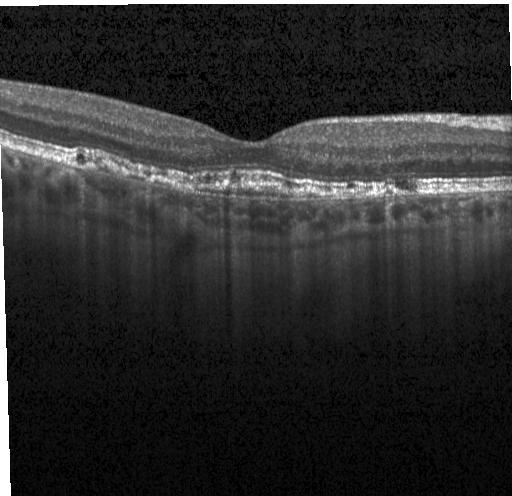 Optical coherence tomography B-scan. Spectral-domain optical coherence tomography. Through the macula — Finding: CNV.